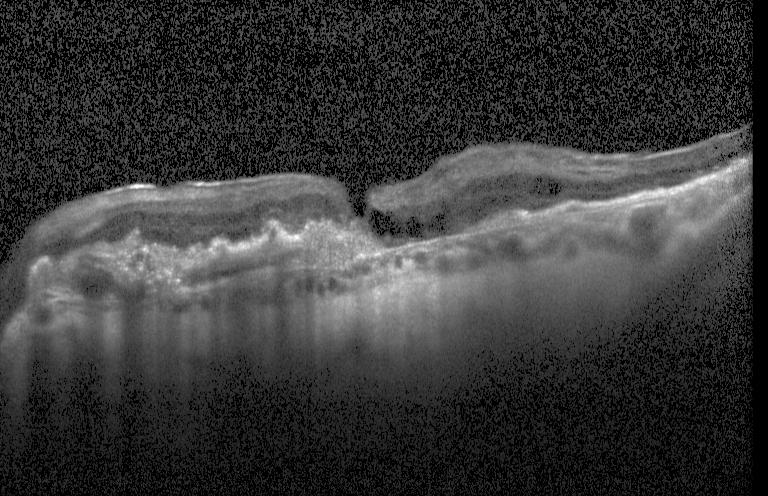

This B-scan demonstrates a choroidal neovascular membrane.